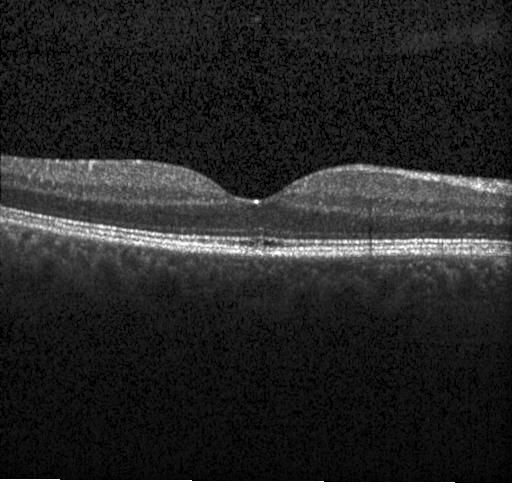
This B-scan demonstrates no evidence of choroidal neovascularization, diabetic macular edema, or drusen.